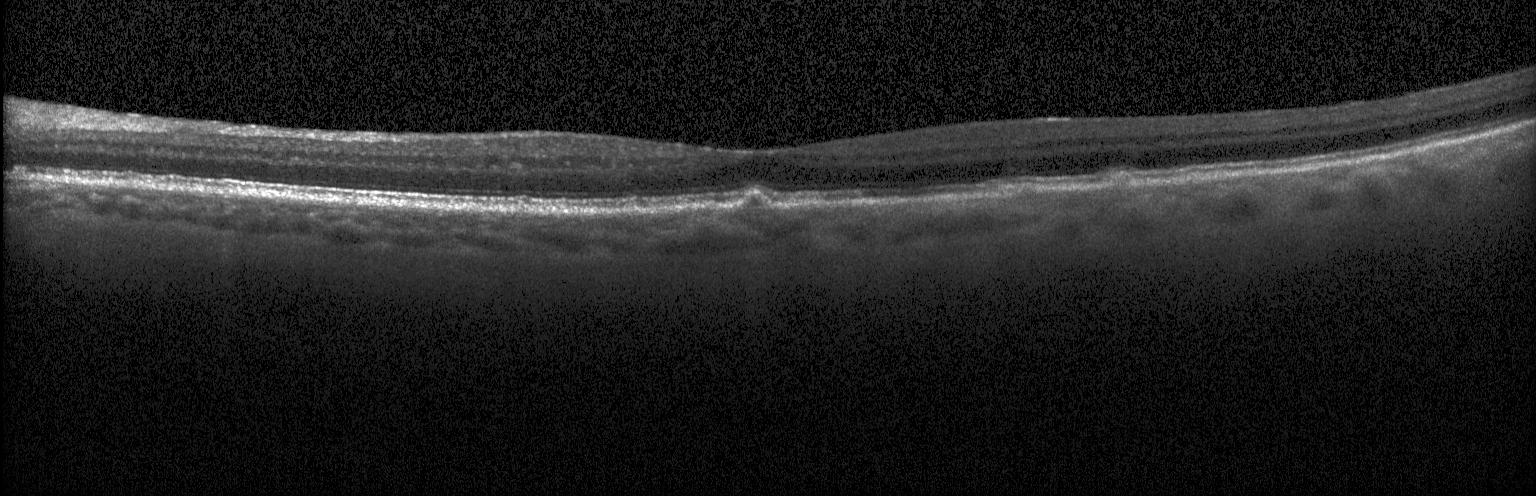
Retinal OCT cross-section · spectral-domain OCT.
Finding: drusen.